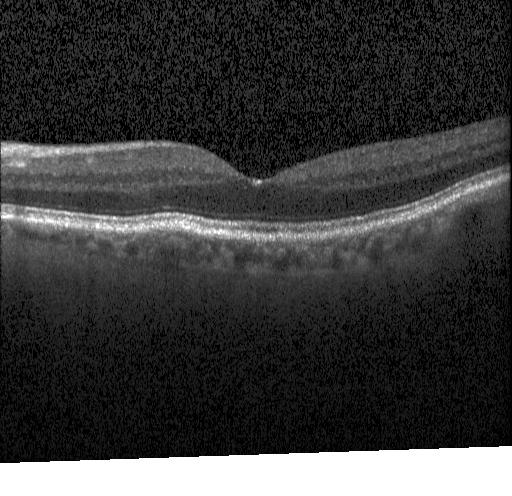 Macular OCT demonstrating neither choroidal neovascularization, diabetic macular edema, nor drusen.